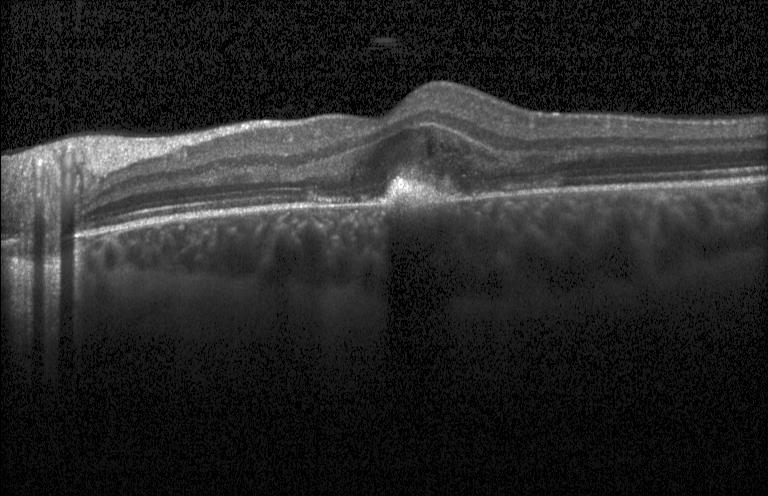
Spectral-domain OCT · Heidelberg Spectralis · optical coherence tomography B-scan
Choroidal neovascularization (CNV).